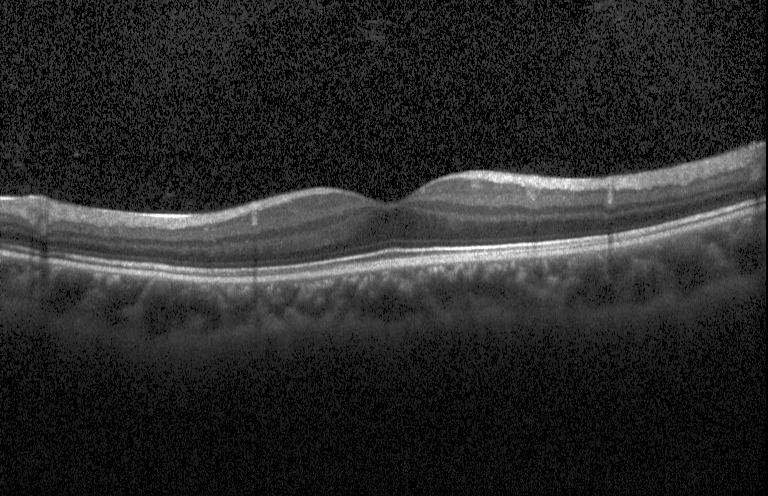

Retinal OCT B-scan. Finding: no evidence of choroidal neovascularization, diabetic macular edema, or drusen.